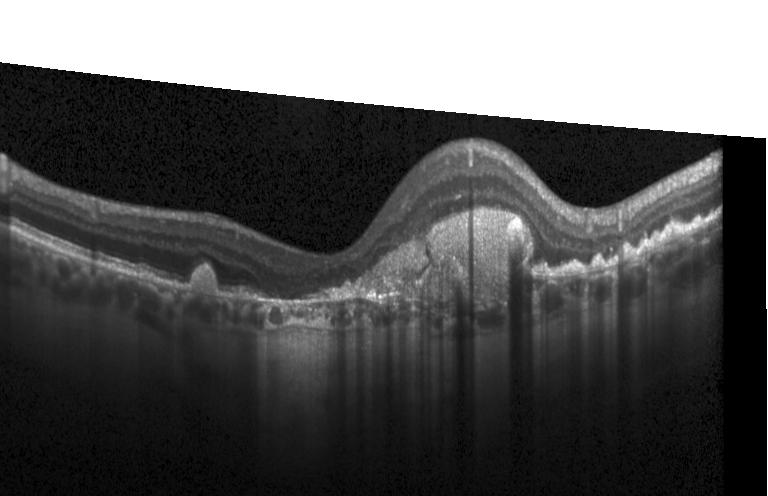
Spectral-domain OCT. Retinal OCT cross-section. Fovea-centered. Heidelberg Spectralis OCT system
This B-scan demonstrates CNV.